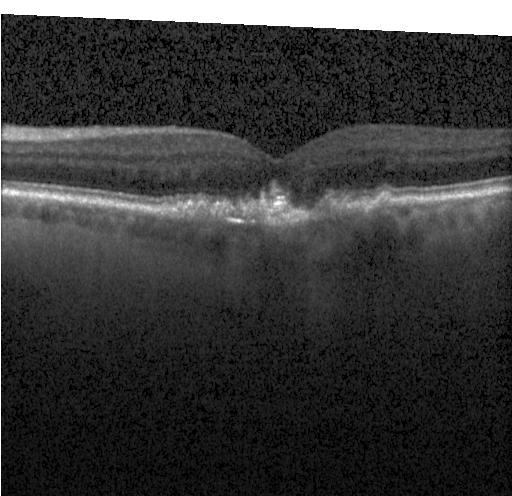
Impression: a choroidal neovascular membrane.